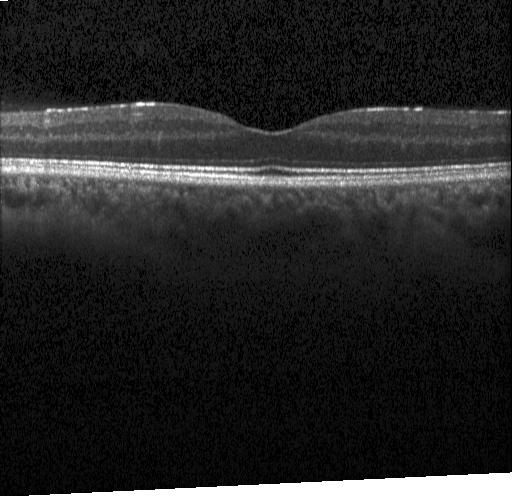 SD-OCT; Heidelberg Spectralis OCT system; horizontal scan through the fovea; optical coherence tomography scan. Finding: no CNV, DME, or drusen.